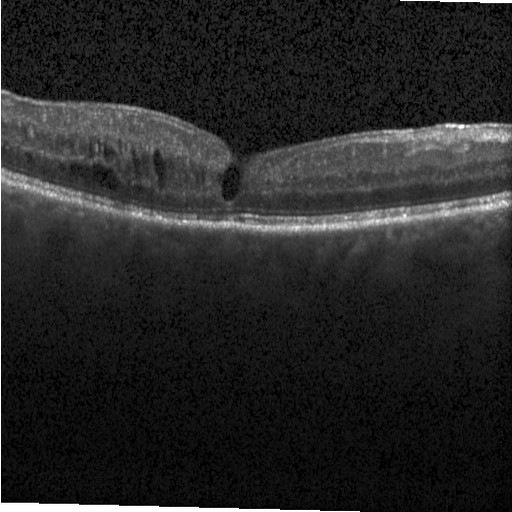
Heidelberg Spectralis; optical coherence tomography B-scan. Dx: diabetic macular edema.